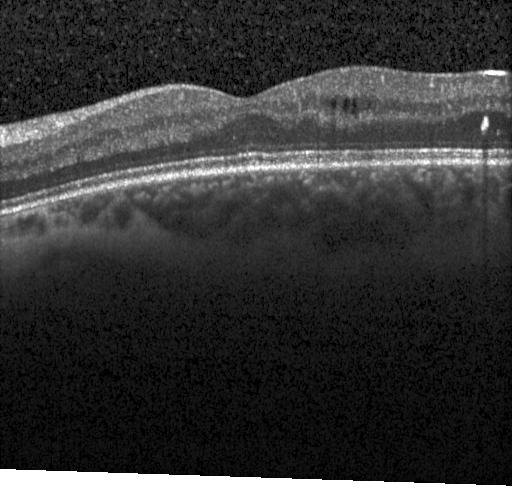 Spectral-domain OCT B-scan: DME.